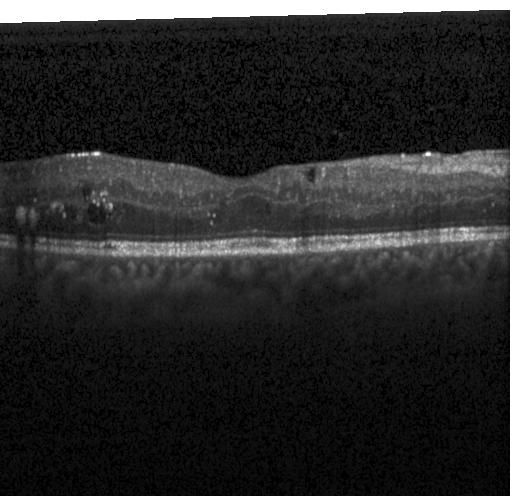

OCT line scan, fovea-centered, acquired on a Heidelberg Spectralis, spectral-domain optical coherence tomography.
OCT finding: diabetic macular edema.